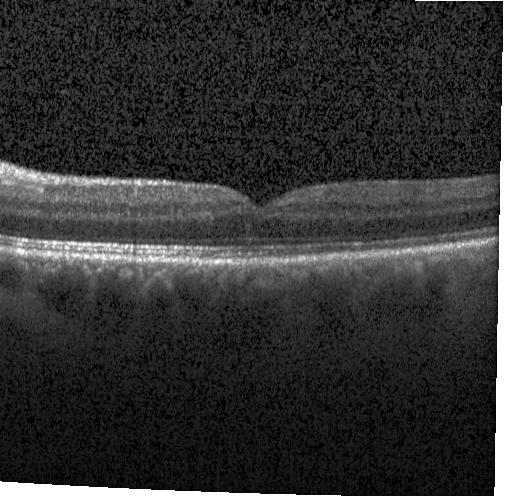

Spectral-domain optical coherence tomography, acquired on a Heidelberg Spectralis, OCT B-scan, through the macula.
Finding: no CNV, no DME, and no drusen.